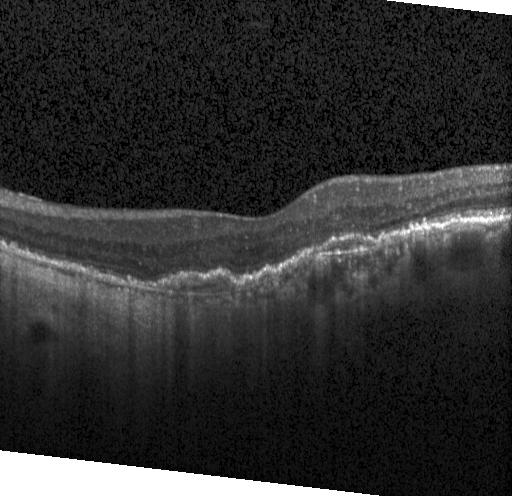
SD-OCT. Acquired on a Heidelberg Spectralis. Optical coherence tomography scan. Through the macula
OCT finding: choroidal neovascularization.